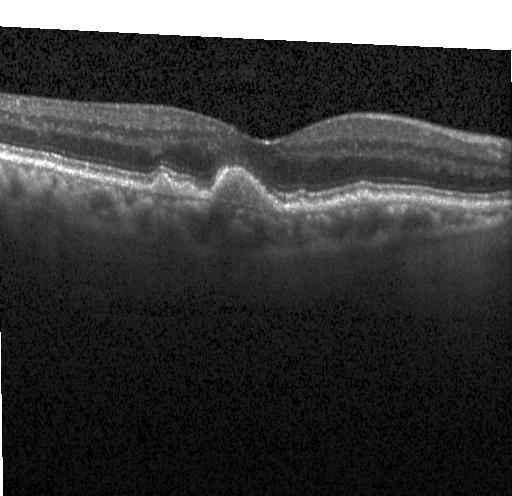 Heidelberg Spectralis; optical coherence tomography scan. Multiple drusen.